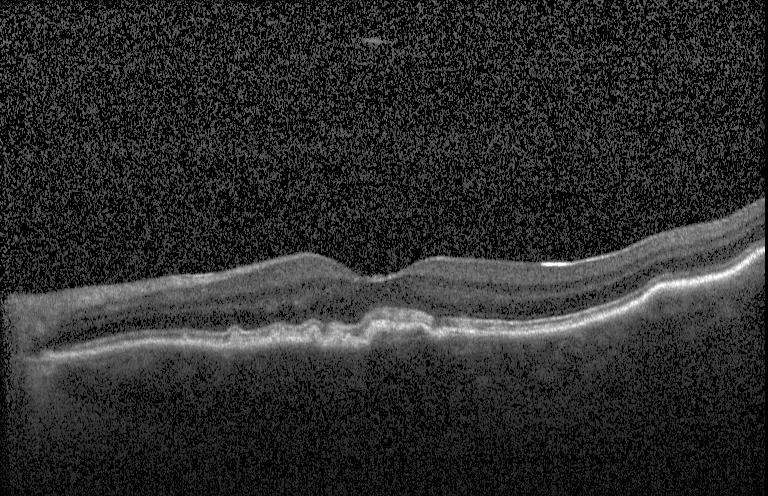
Spectral-domain optical coherence tomography. Retinal OCT B-scan. Horizontal scan through the fovea. Heidelberg Spectralis — This B-scan demonstrates multiple drusen.